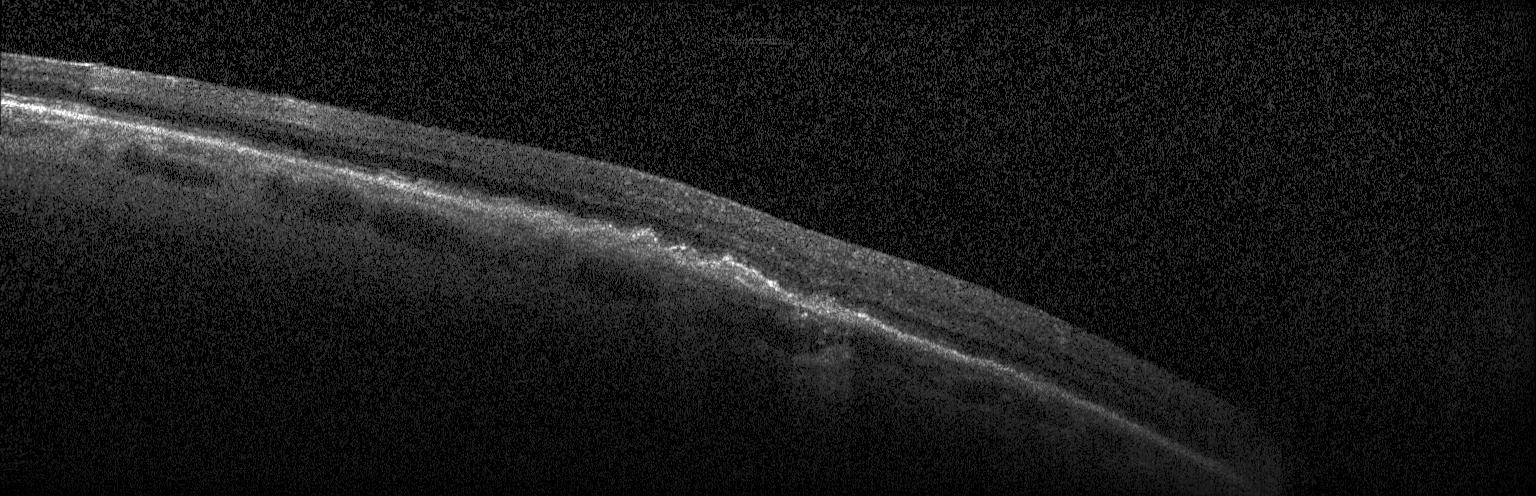 Retinal OCT cross-section. Heidelberg Spectralis. Diagnosis: a choroidal neovascular membrane.